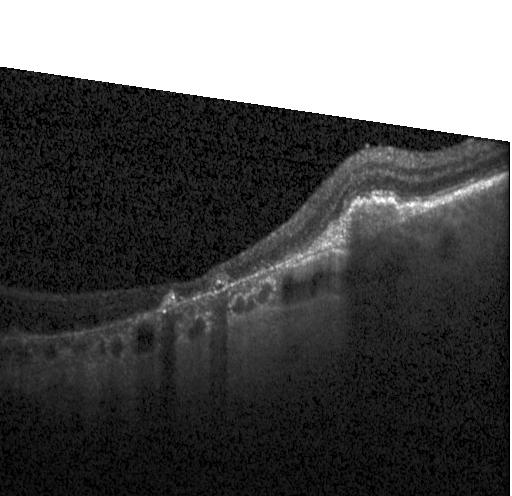 Retinal OCT cross-section. Centered on the fovea. SD-OCT
Diagnosis: choroidal neovascularization.